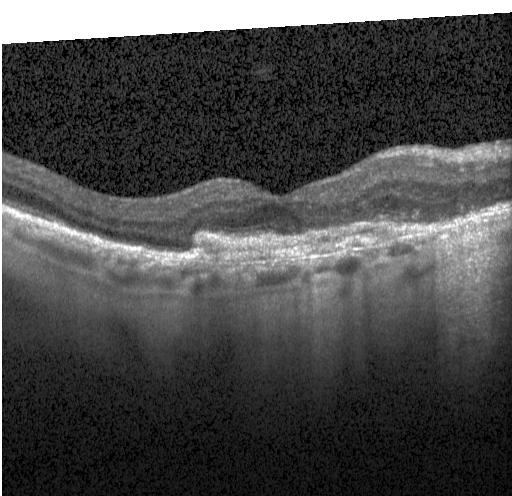 Heidelberg Spectralis, SD-OCT, horizontal scan through the fovea, OCT B-scan. Finding: choroidal neovascularization.